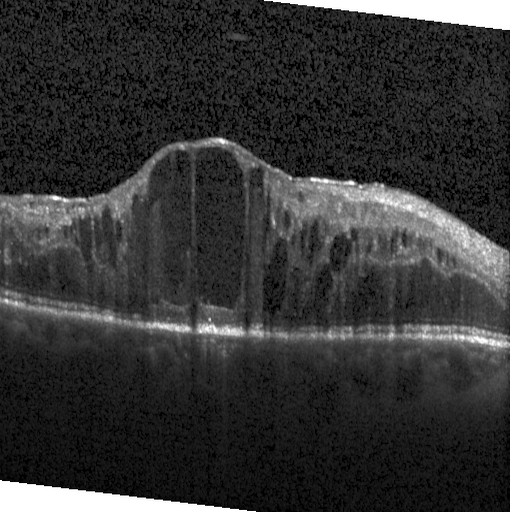 Retinal OCT B-scan.
Macular OCT: diabetic macular edema.